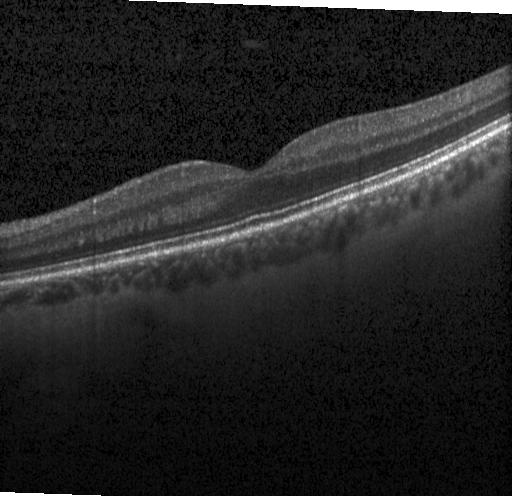
Impression: no choroidal neovascularization, diabetic macular edema, or drusen.